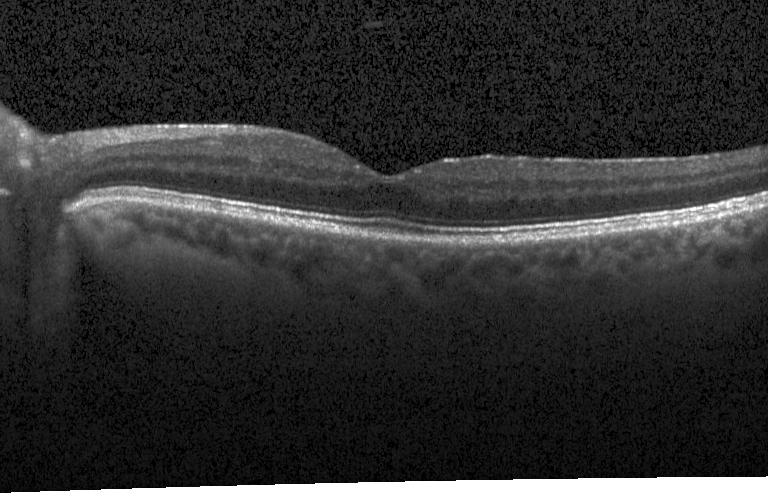

Dx: no choroidal neovascularization, diabetic macular edema, or drusen.